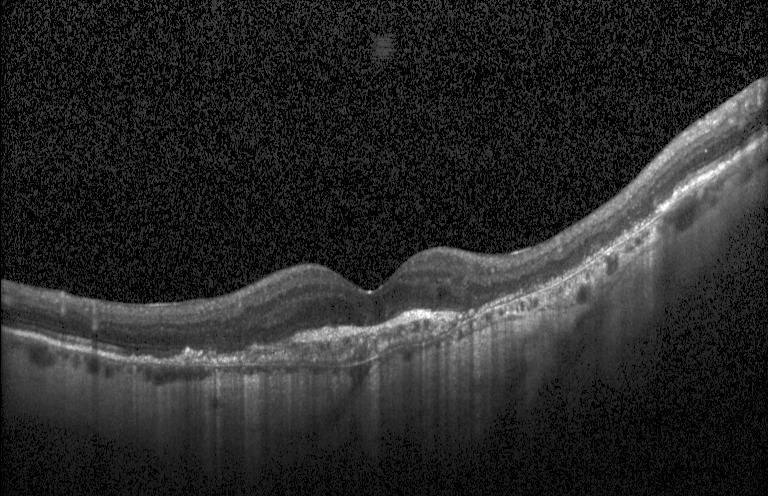
Spectral-domain OCT B-scan: choroidal neovascularization.